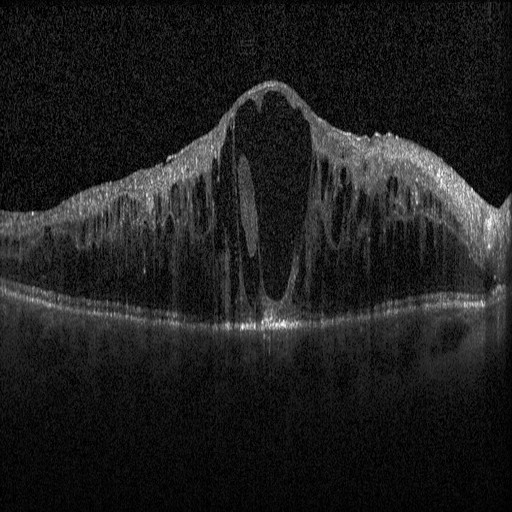

This B-scan demonstrates diabetic macular edema (DME).